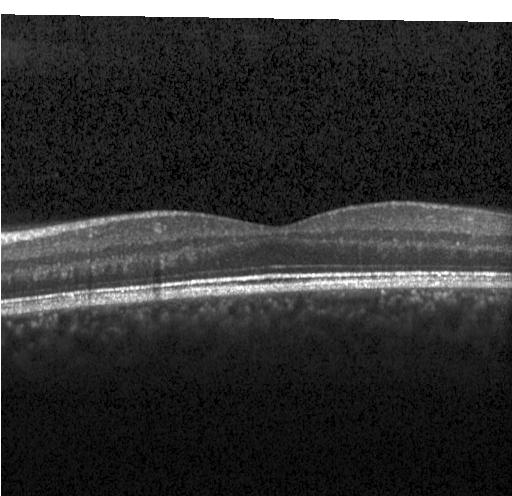
The scan shows no choroidal neovascularization, no diabetic macular edema, and no drusen.